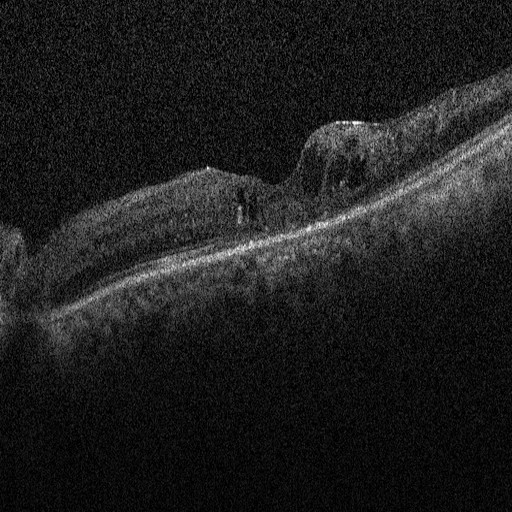 OCT line scan; spectral-domain OCT.
OCT finding: diabetic macular edema.